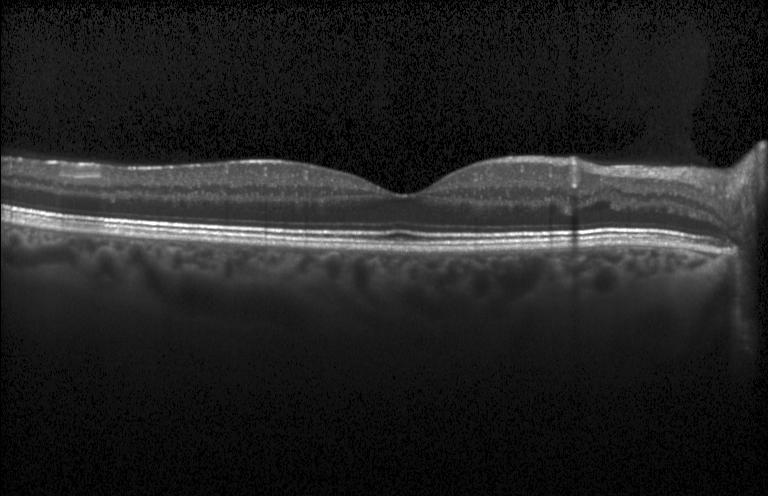
Macular OCT demonstrating no choroidal neovascularization, no diabetic macular edema, and no drusen.